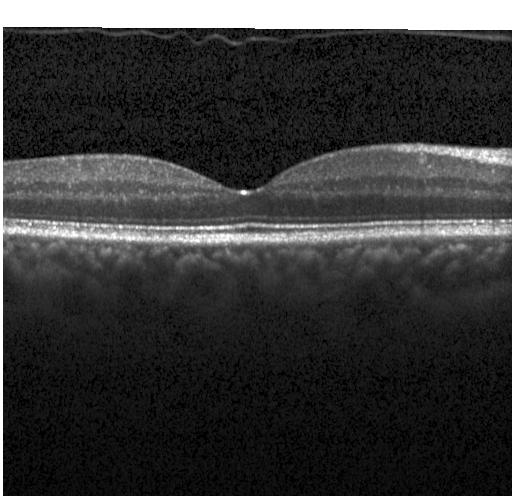 Retinal OCT cross-section, SD-OCT.
Diagnosis: neither choroidal neovascularization, diabetic macular edema, nor drusen.